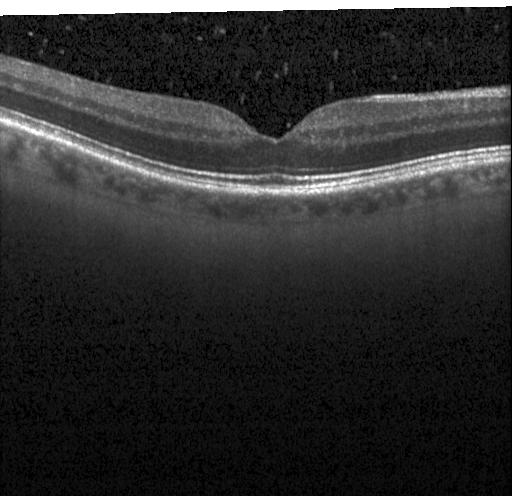

OCT B-scan. Heidelberg Spectralis. Horizontal scan through the fovea — Macular OCT: no choroidal neovascularization, no diabetic macular edema, and no drusen.